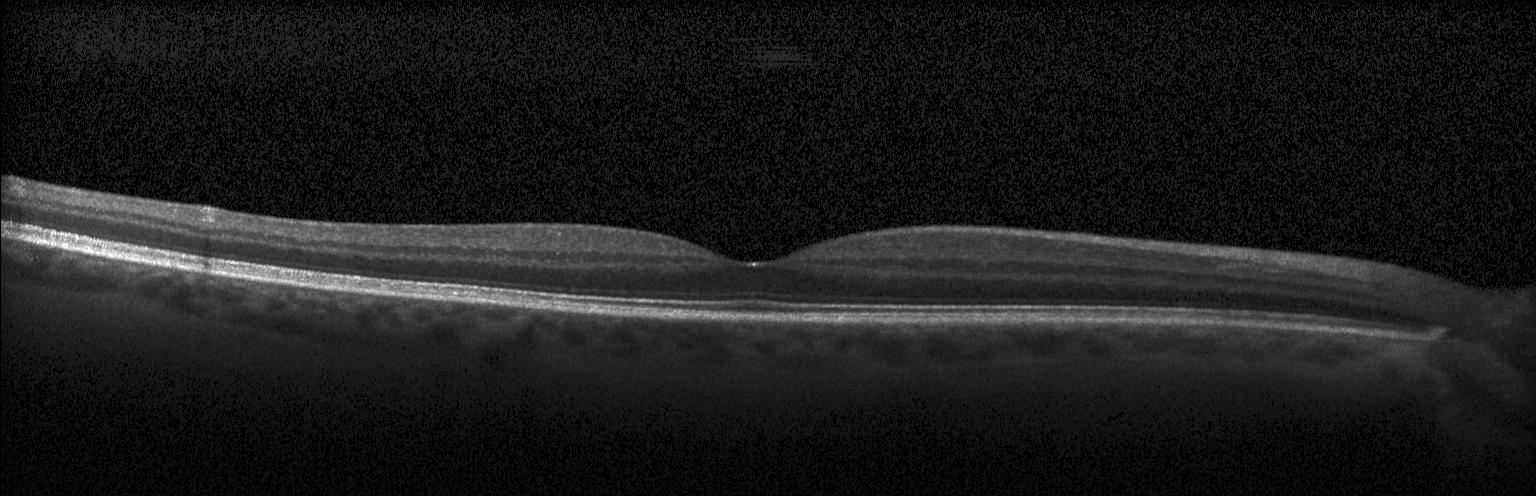

Spectral-domain OCT. Optical coherence tomography scan. Heidelberg Spectralis. Horizontal scan through the fovea
The scan shows no choroidal neovascularization, diabetic macular edema, or drusen.